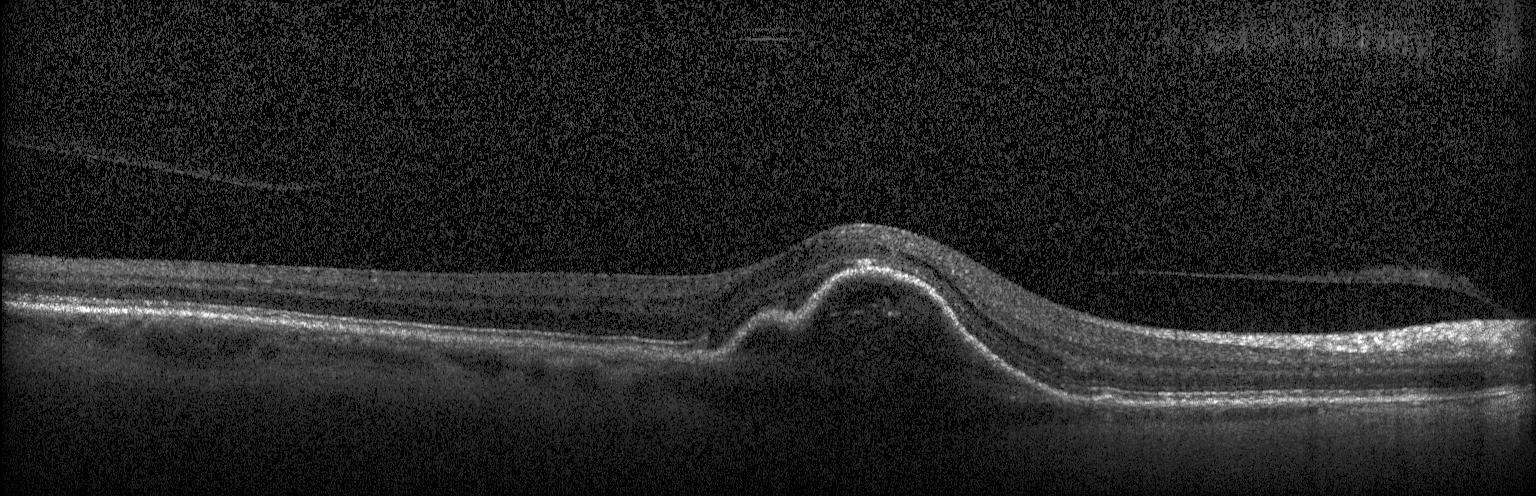

The scan shows CNV.